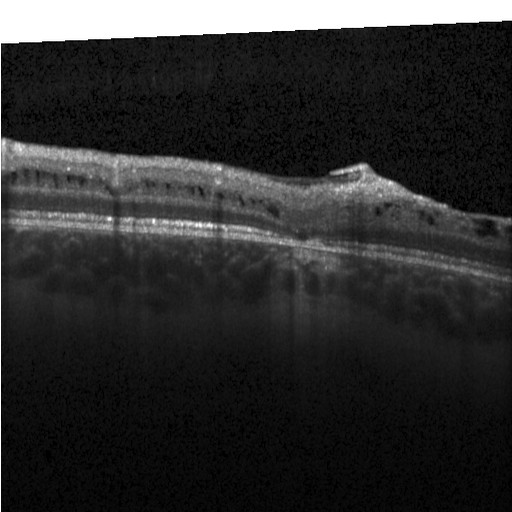 Retinal OCT B-scan
Assessment: DME.